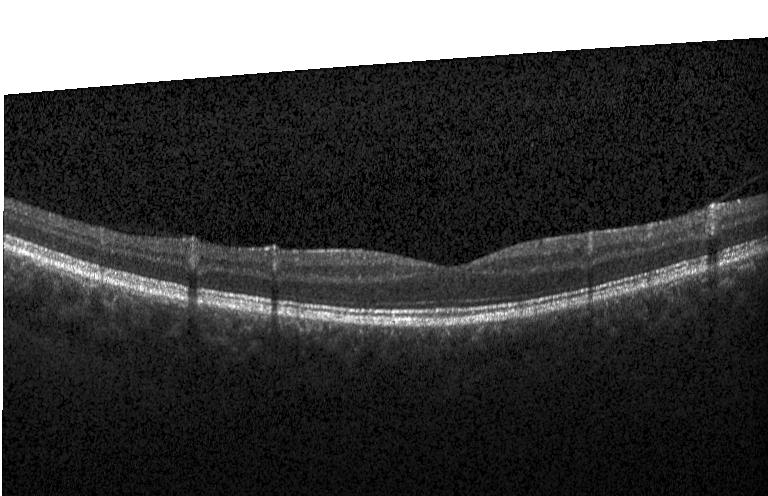 Optical coherence tomography B-scan — This B-scan demonstrates no choroidal neovascularization, diabetic macular edema, or drusen.